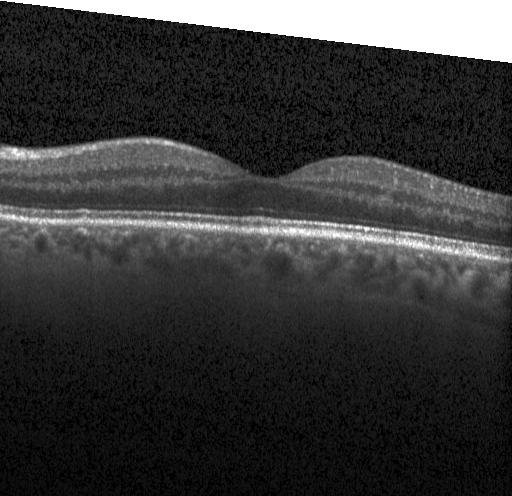
OCT line scan; macular scan; Heidelberg Spectralis; spectral-domain OCT
Finding: no evidence of choroidal neovascularization, diabetic macular edema, or drusen.